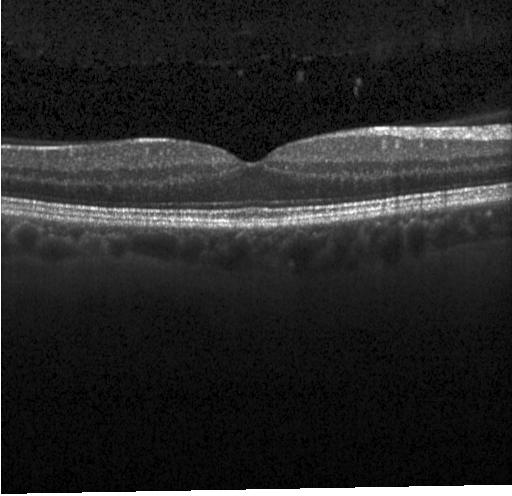

Optical coherence tomography scan.
Finding: no evidence of CNV, DME, or drusen.